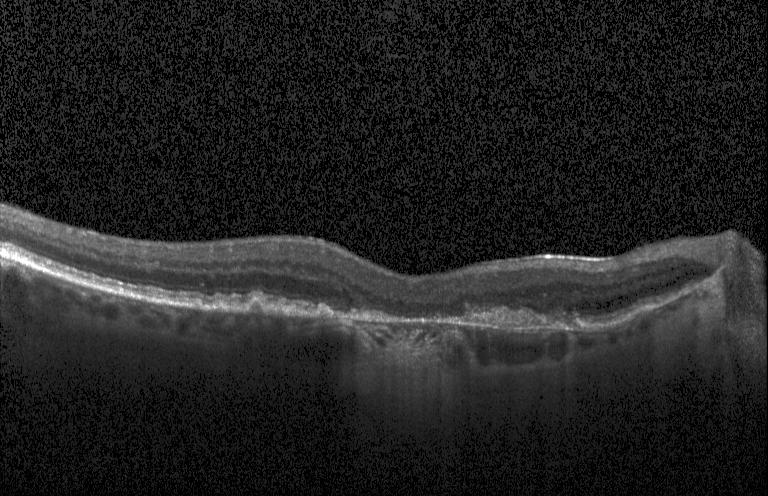

OCT B-scan · centered on the fovea · instrument: Heidelberg Spectralis.
Macular OCT: choroidal neovascularization (CNV).